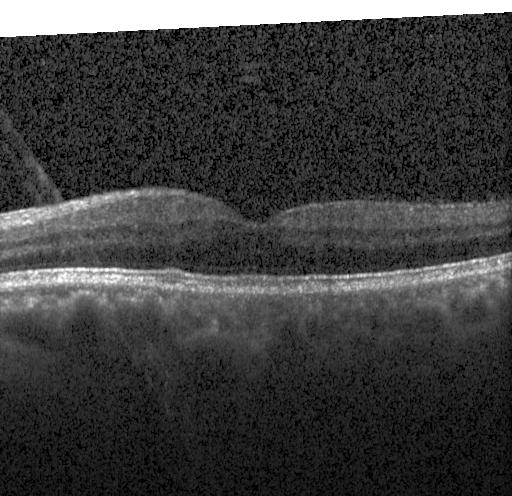 Instrument: Heidelberg Spectralis, retinal OCT B-scan, spectral-domain OCT, horizontal scan through the fovea
Finding: no choroidal neovascularization, diabetic macular edema, or drusen.